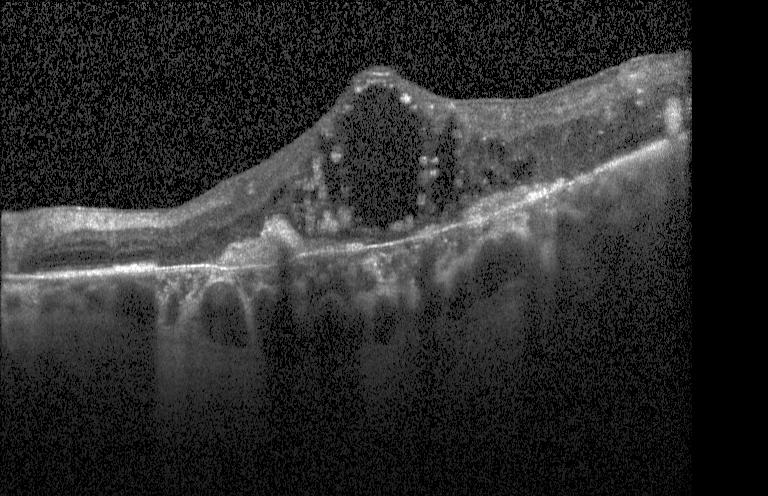 Spectral-domain OCT B-scan: a choroidal neovascular membrane.